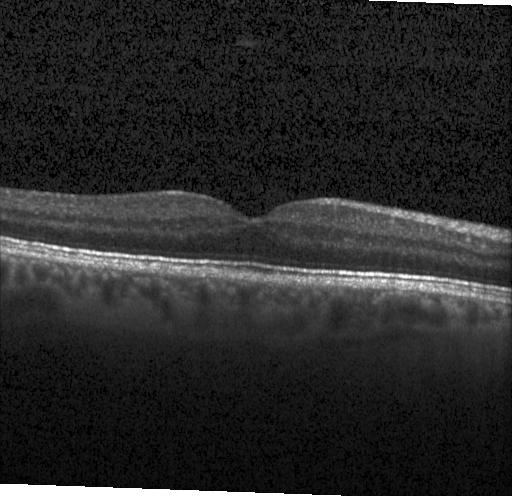 Through the macula · Heidelberg Spectralis · retinal OCT B-scan · SD-OCT
Finding: no evidence of CNV, DME, or drusen.